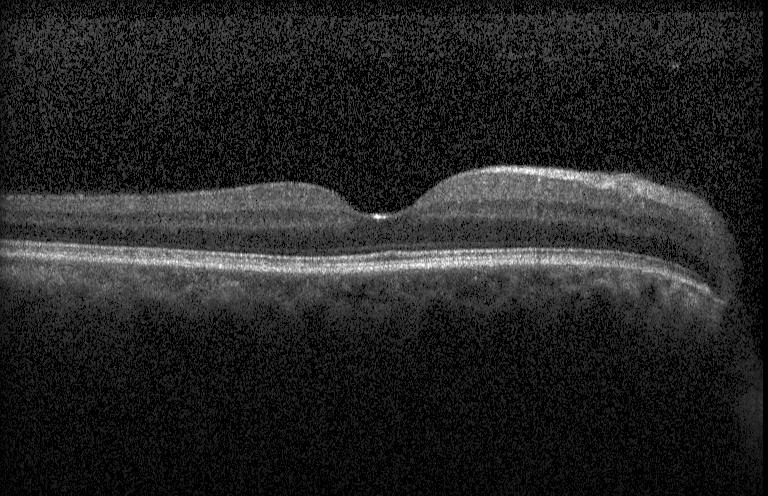

Heidelberg Spectralis OCT system · retinal OCT cross-section.
Impression: no choroidal neovascularization, diabetic macular edema, or drusen.